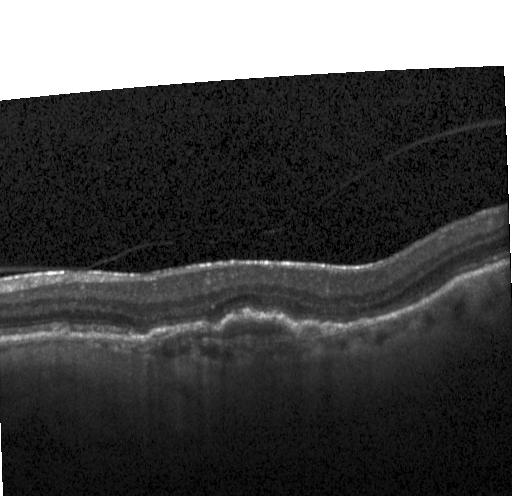
Retinal OCT cross-section, SD-OCT, acquired on a Heidelberg Spectralis. Diagnosis: a choroidal neovascular membrane.